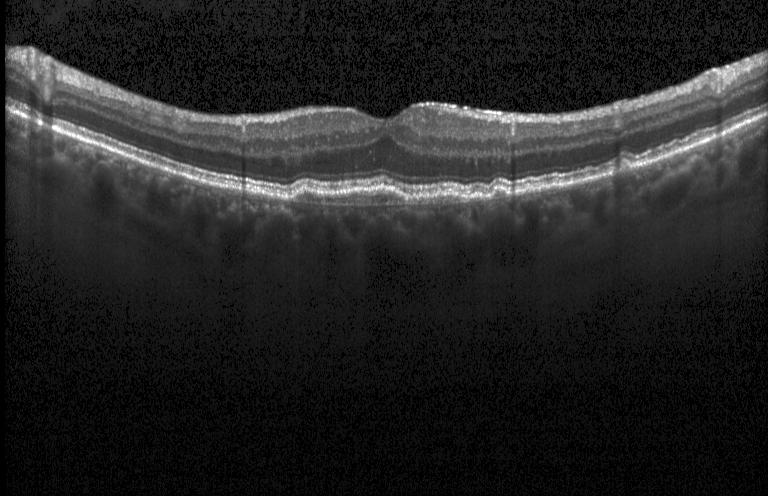 The scan shows CNV.